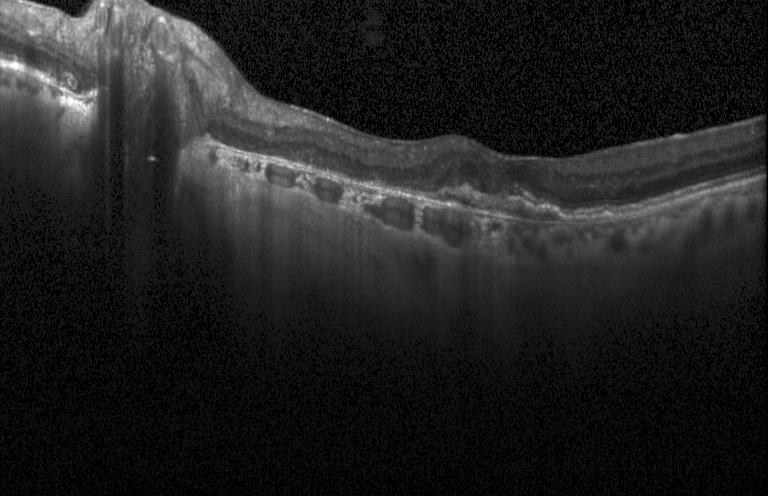 OCT line scan.
Dx: a choroidal neovascular membrane.